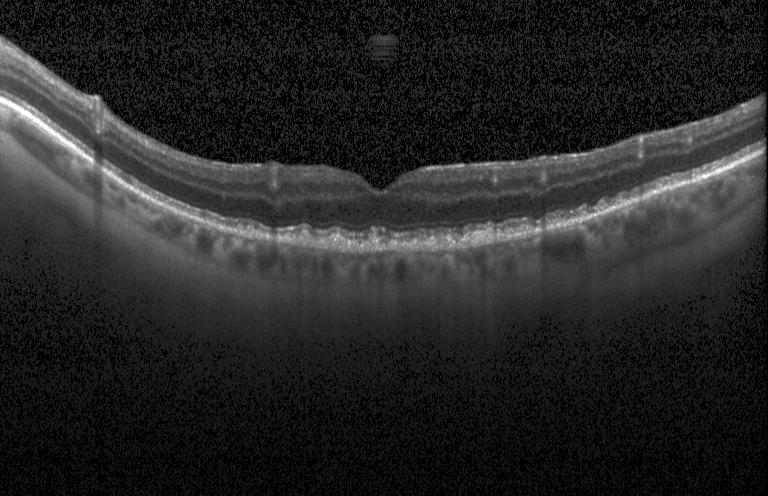
OCT B-scan
Sub-RPE drusenoid deposits.